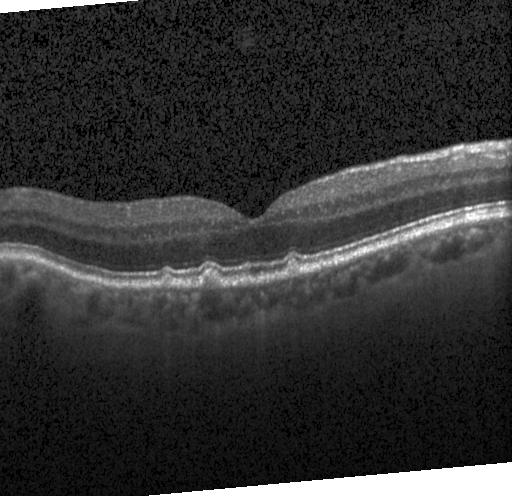

Optical coherence tomography B-scan; through the macula. Diagnosis: drusen.